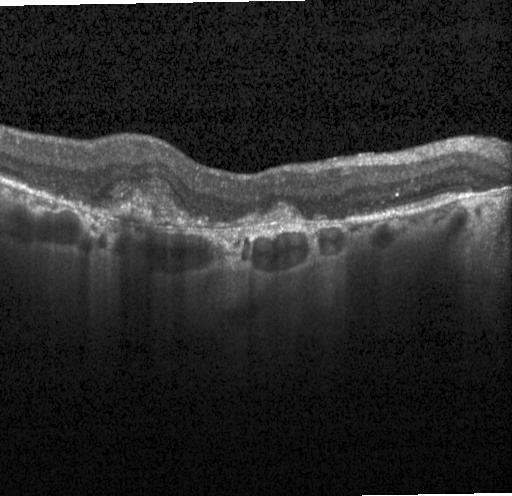
Impression: choroidal neovascularization.